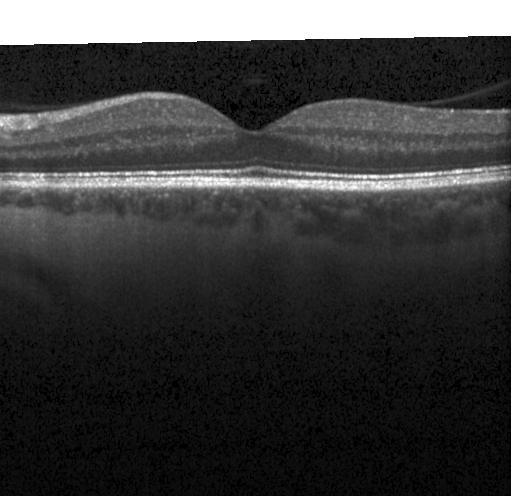

This B-scan demonstrates neither CNV, DME, nor drusen.